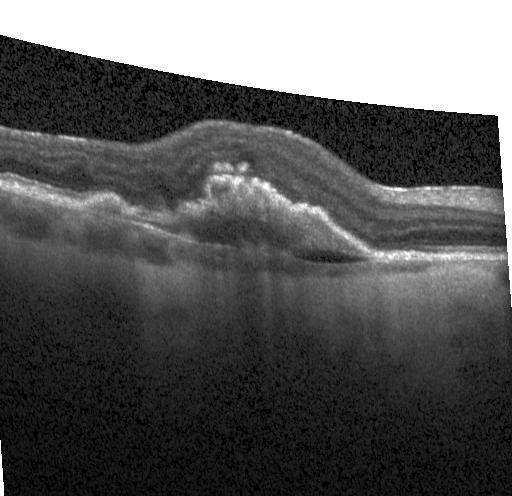 The scan shows a choroidal neovascular membrane.